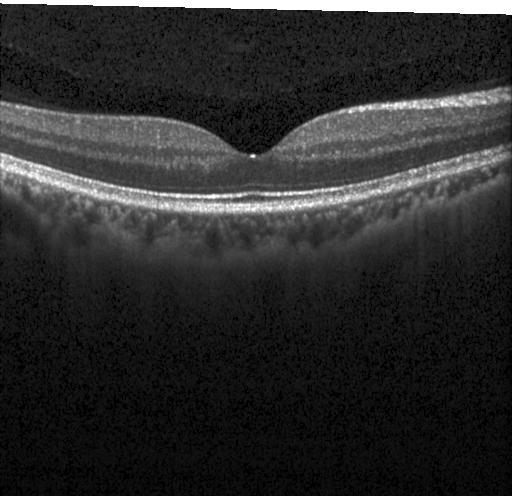 Optical coherence tomography B-scan · Heidelberg Spectralis. OCT finding: no evidence of choroidal neovascularization, diabetic macular edema, or drusen.